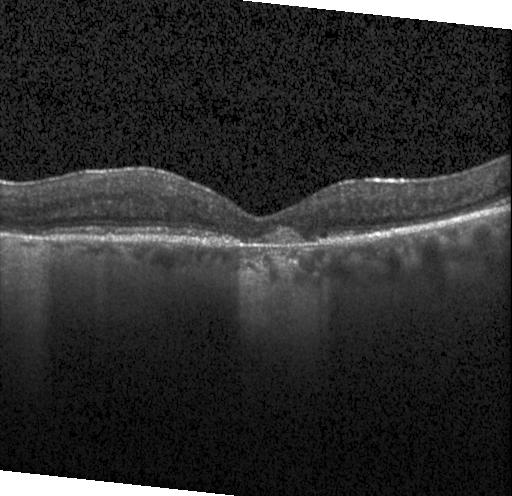

Spectral-domain OCT · optical coherence tomography B-scan
Impression: CNV.